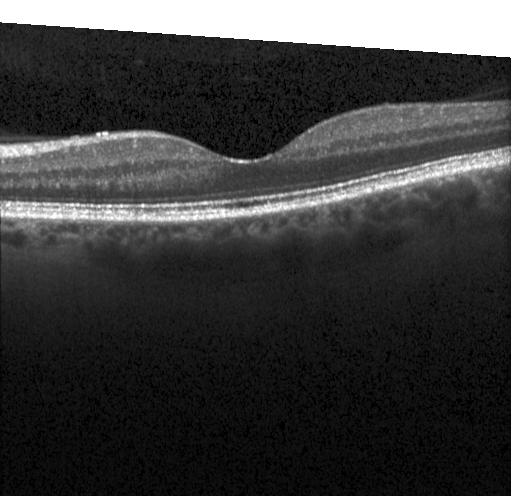
Macular OCT demonstrating no choroidal neovascularization, diabetic macular edema, or drusen.